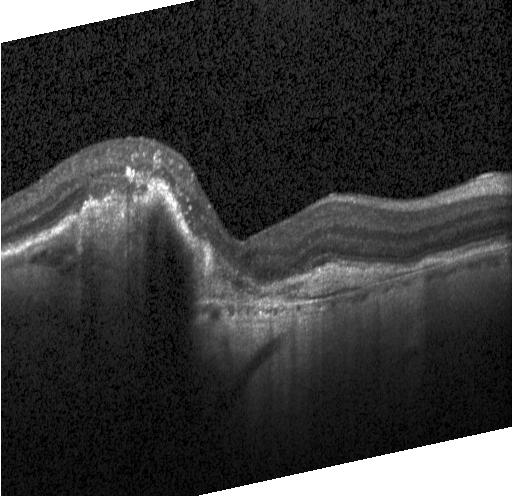

Optical coherence tomography scan · fovea-centered.
Diagnosis: a choroidal neovascular membrane.